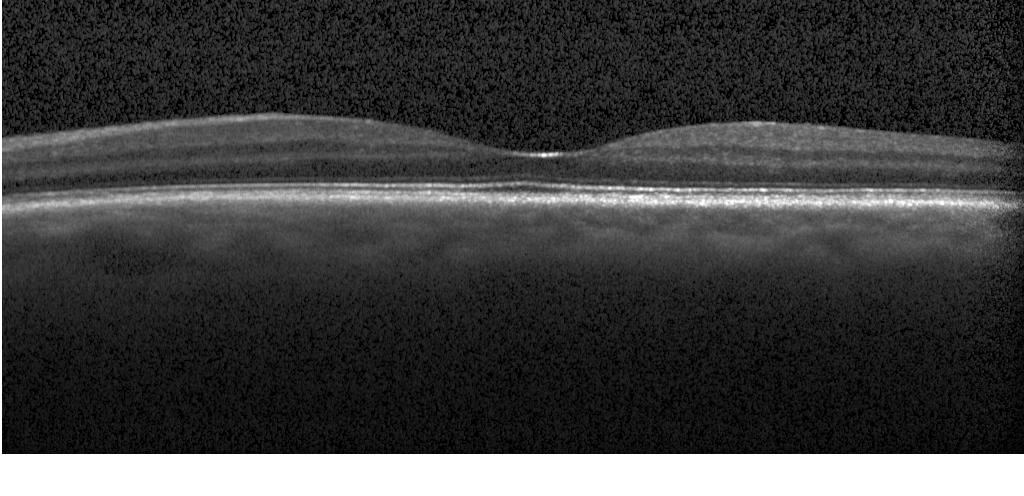
Optical coherence tomography scan — Finding: no evidence of choroidal neovascularization, diabetic macular edema, or drusen.